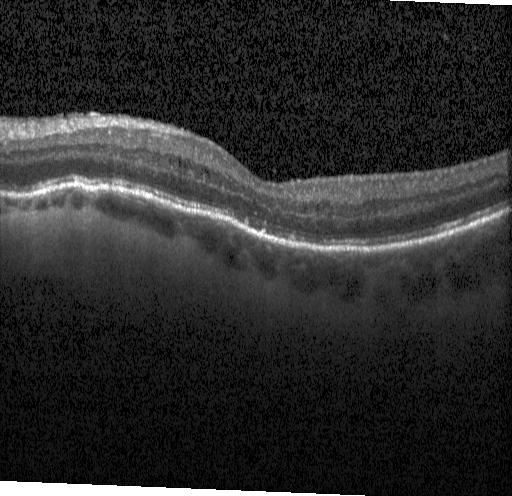
Through the macula. SD-OCT. Heidelberg Spectralis. OCT line scan
Dx: no evidence of choroidal neovascularization, diabetic macular edema, or drusen.